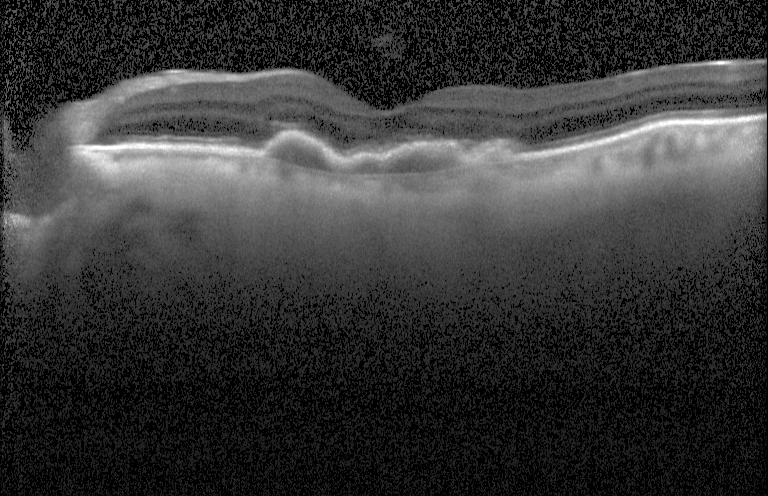

Optical coherence tomography B-scan
Finding: a choroidal neovascular membrane.